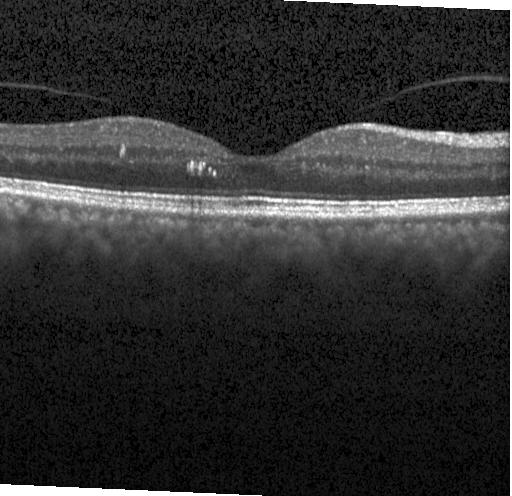 Finding: no choroidal neovascularization, diabetic macular edema, or drusen.